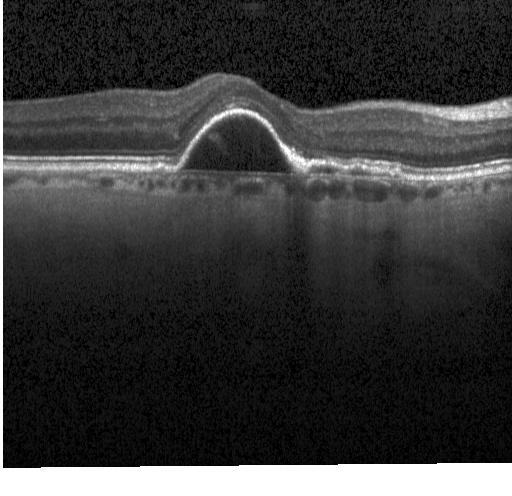 Dx: choroidal neovascularization.